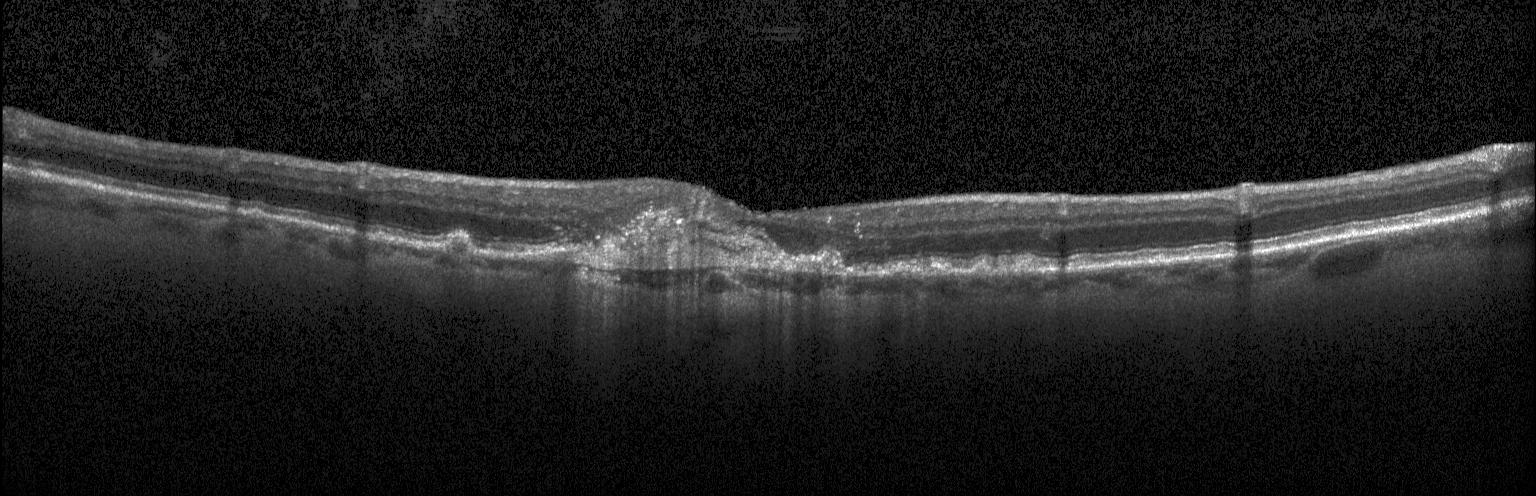 Optical coherence tomography scan.
Diagnosis: a choroidal neovascular membrane.